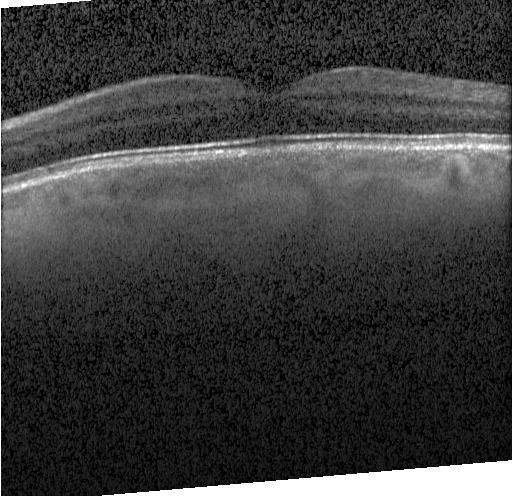

OCT scan showing no choroidal neovascularization, no diabetic macular edema, and no drusen.